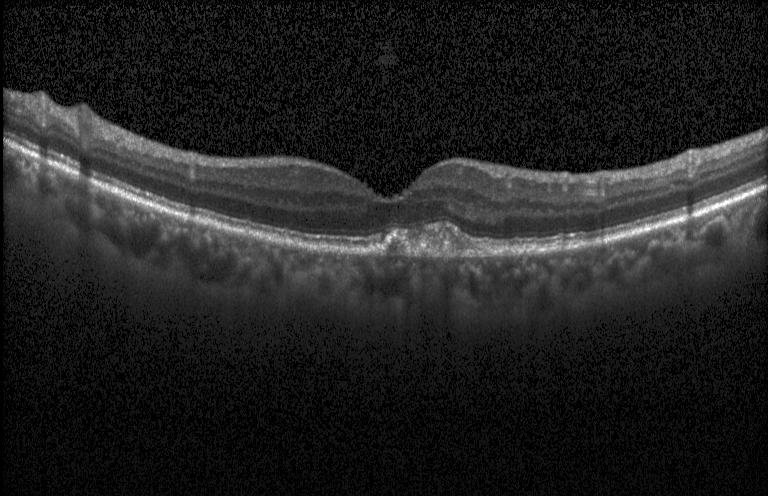

Retinal OCT cross-section. This B-scan demonstrates multiple drusen.